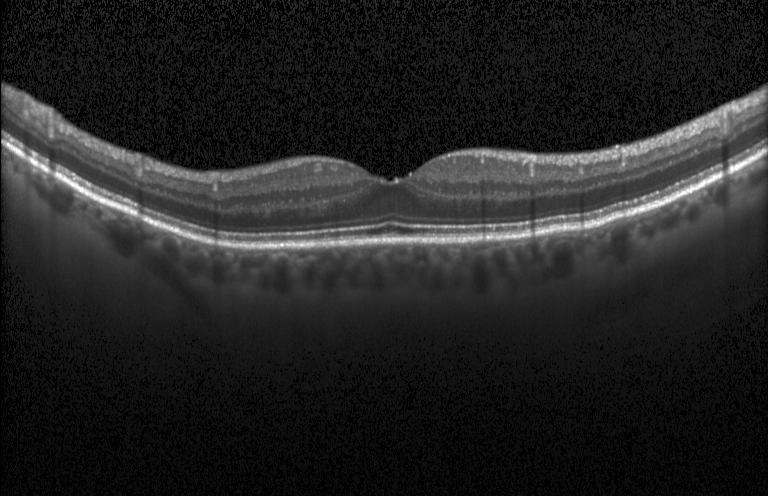
Dx: no CNV, DME, or drusen.